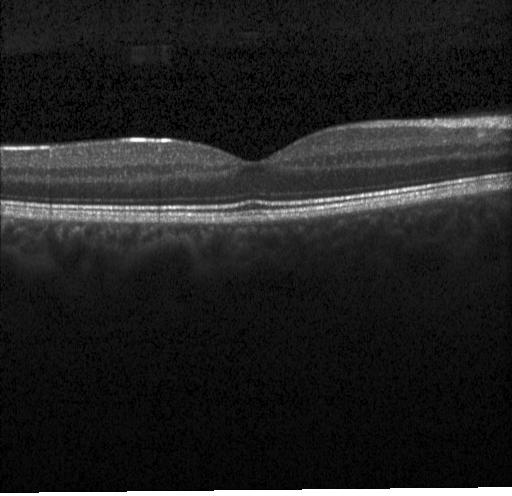 Diagnosis: no evidence of CNV, DME, or drusen.